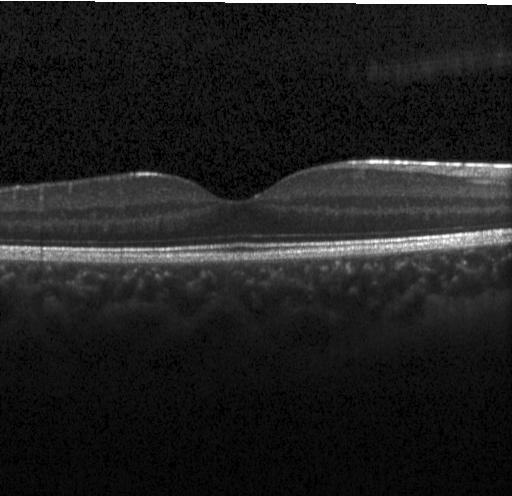

Dx: no evidence of CNV, DME, or drusen.